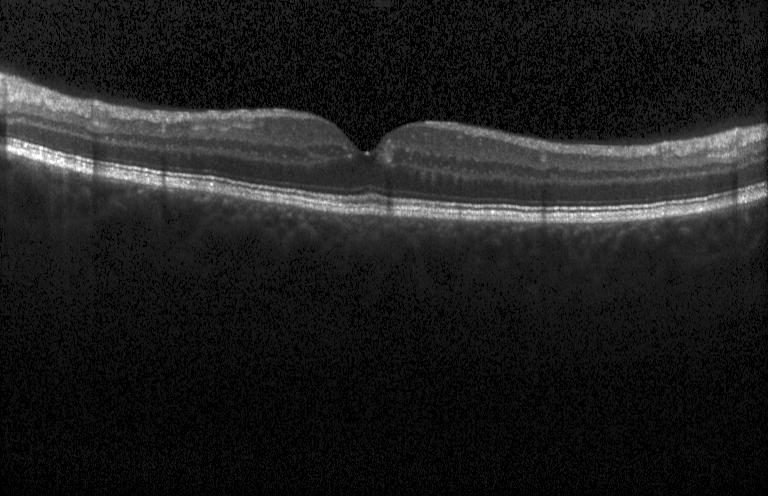
Spectral-domain optical coherence tomography · optical coherence tomography scan — Impression: neither CNV, DME, nor drusen.